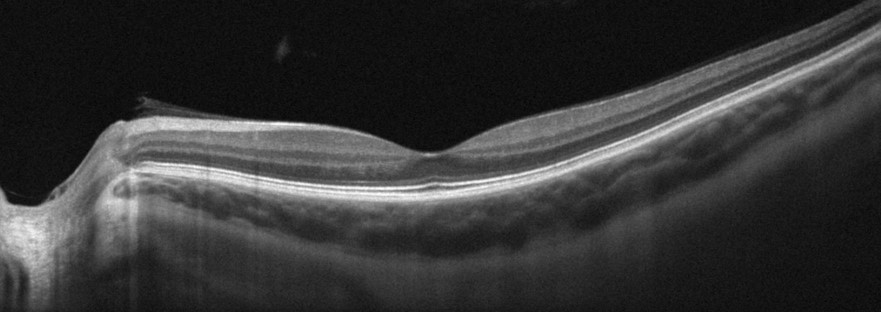 Retinal OCT B-scan
Finding: no evidence of AMD, DME, ERM, RAO, RVO, or VID.